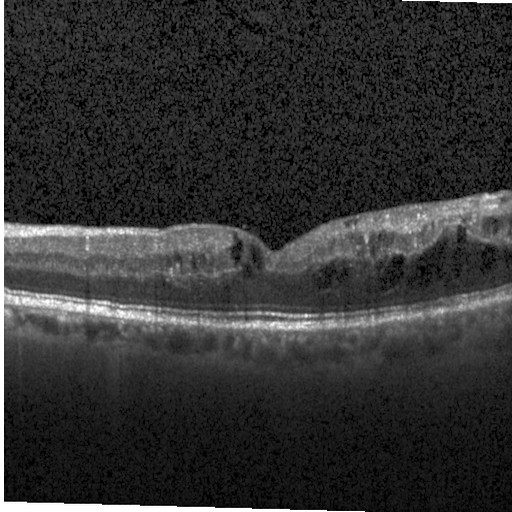
OCT line scan
Impression: diabetic macular edema.